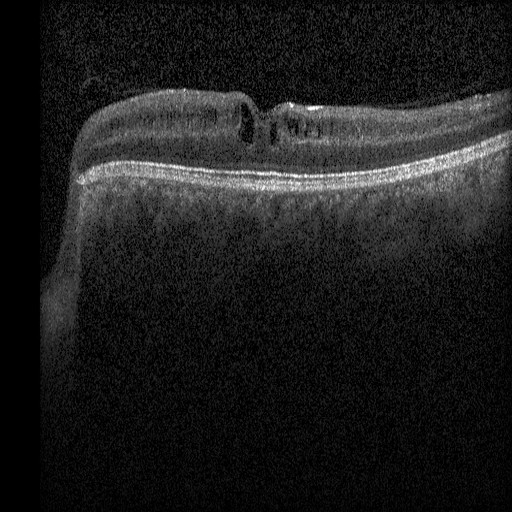 Assessment: diabetic macular edema (DME).